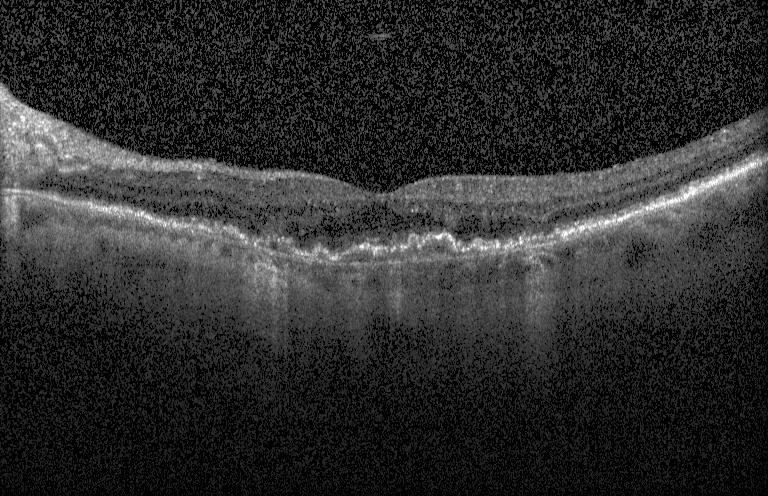 OCT finding: choroidal neovascularization (CNV).